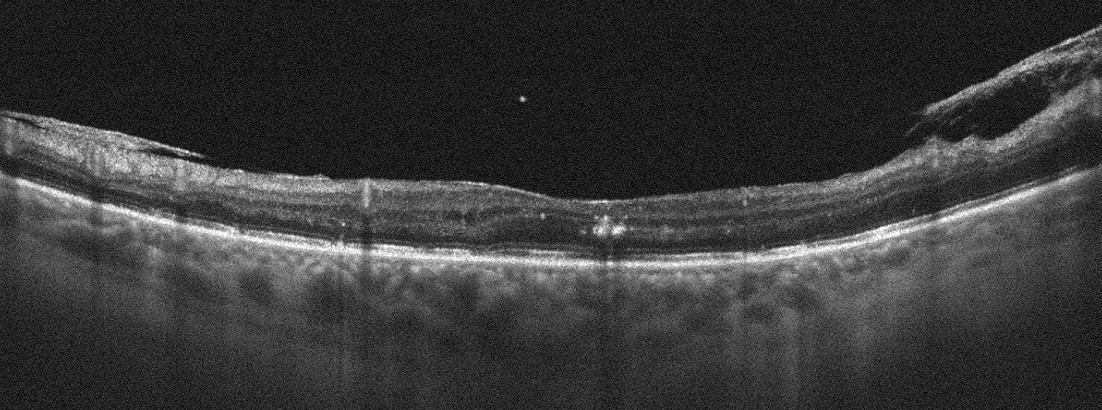
Retinal OCT cross-section
Impression: diabetic macular edema (DME).